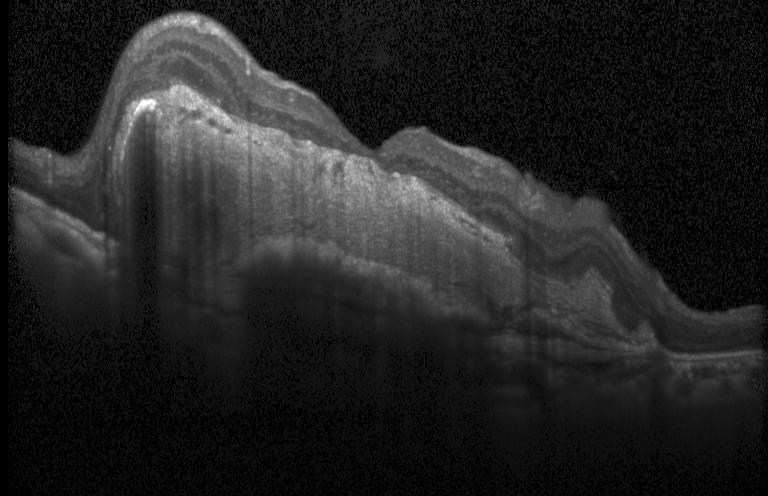 Impression: choroidal neovascularization.